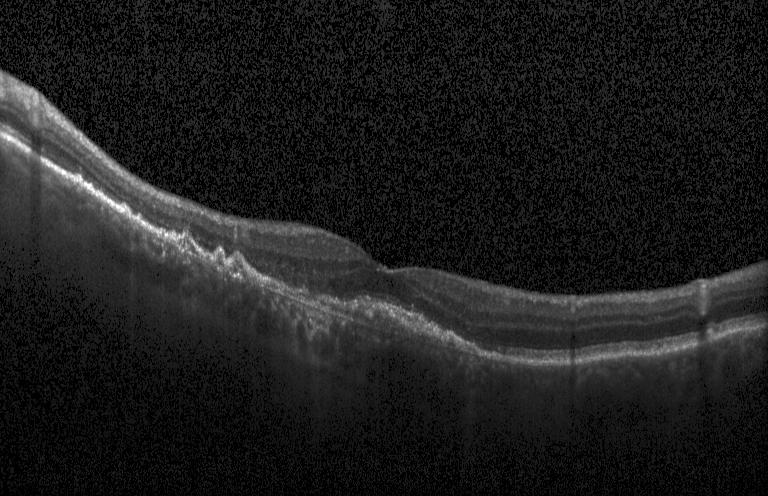 OCT line scan; spectral-domain OCT. Diagnosis: a choroidal neovascular membrane.